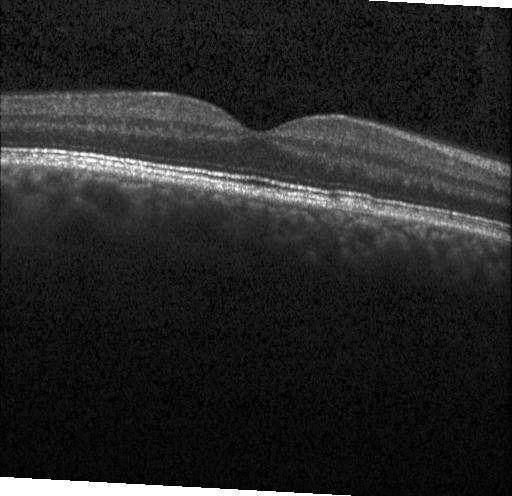
Retinal OCT B-scan · macular scan · SD-OCT. Dx: neither choroidal neovascularization, diabetic macular edema, nor drusen.